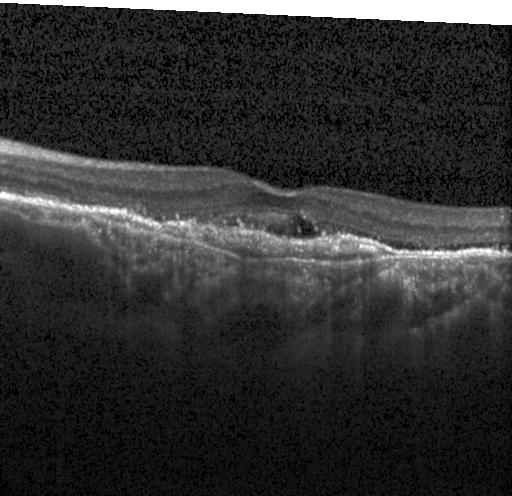 Finding: a choroidal neovascular membrane.